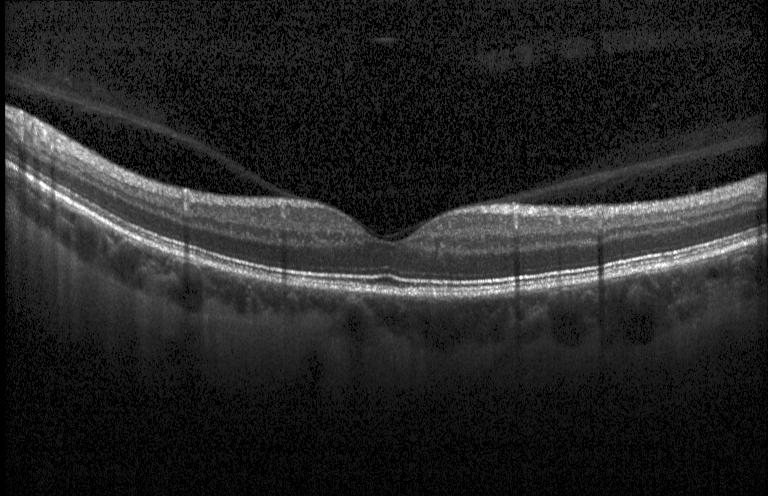 Heidelberg Spectralis OCT system, macular scan, optical coherence tomography B-scan — OCT finding: no choroidal neovascularization, diabetic macular edema, or drusen.